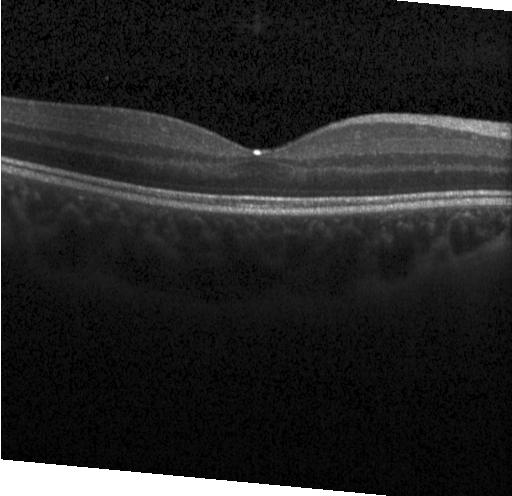
OCT line scan; instrument: Heidelberg Spectralis. Impression: no CNV, DME, or drusen.